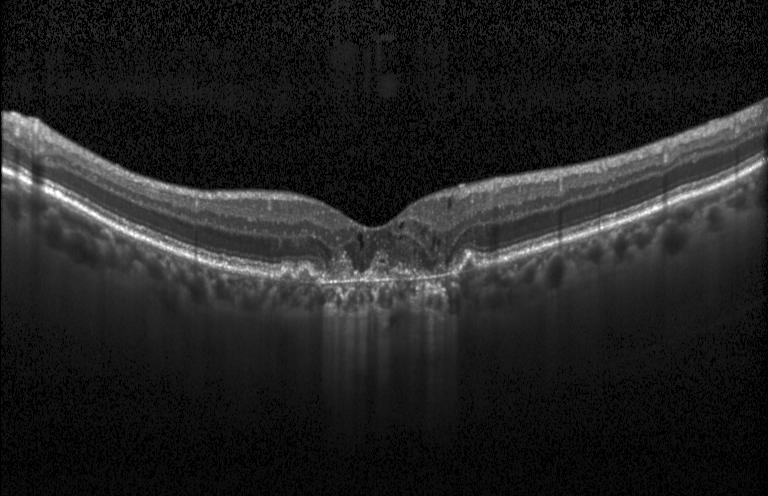 Heidelberg Spectralis OCT system; spectral-domain optical coherence tomography; optical coherence tomography B-scan
The scan shows choroidal neovascularization.